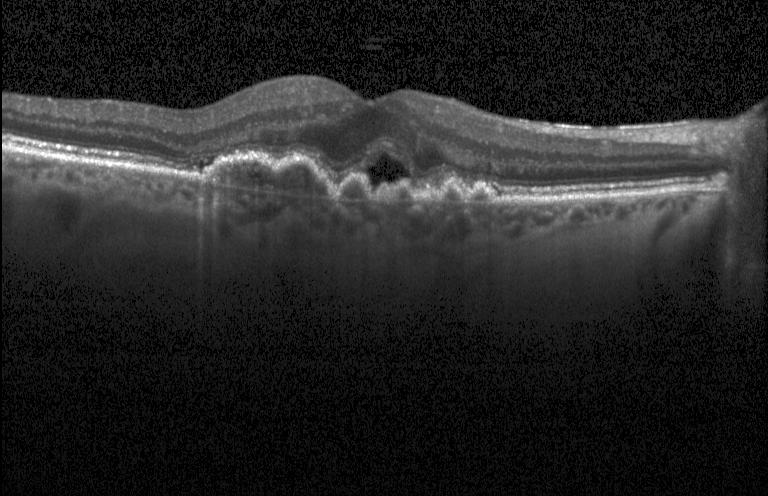
Optical coherence tomography B-scan.
This B-scan demonstrates choroidal neovascularization (CNV).